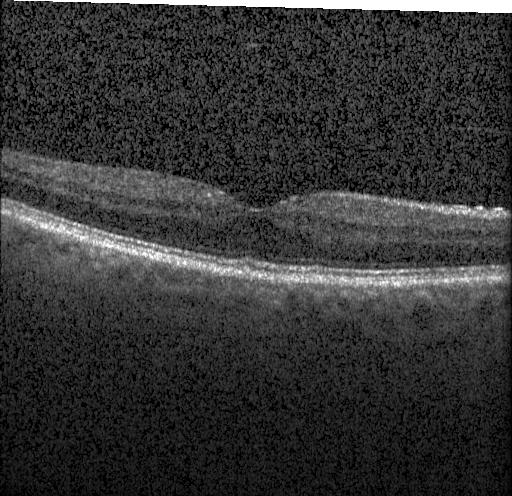
OCT scan showing no choroidal neovascularization, diabetic macular edema, or drusen.